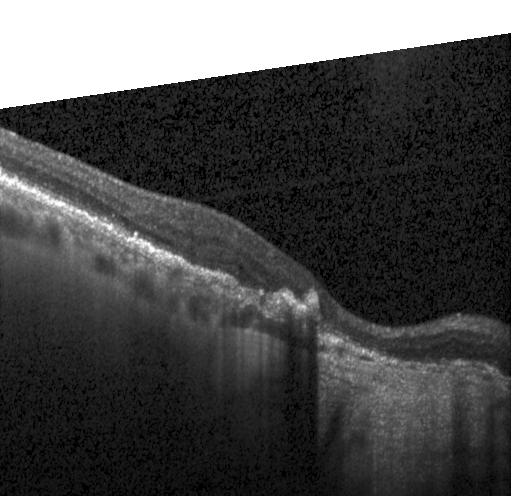
OCT line scan, instrument: Heidelberg Spectralis, SD-OCT, horizontal scan through the fovea.
The scan shows a choroidal neovascular membrane.